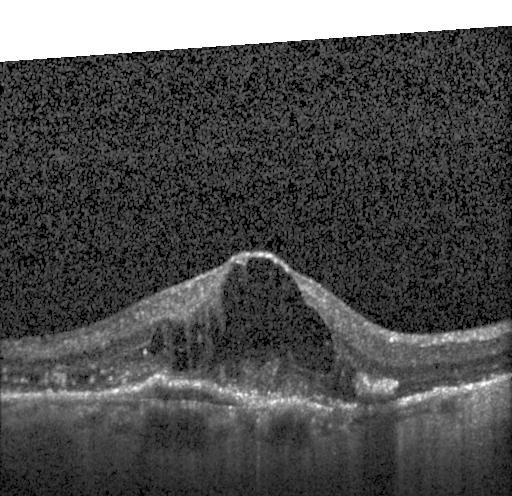
Diagnosis: a choroidal neovascular membrane.